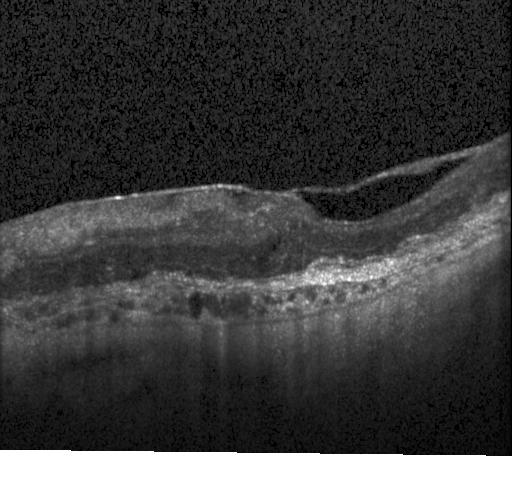 OCT line scan.
Impression: a choroidal neovascular membrane.